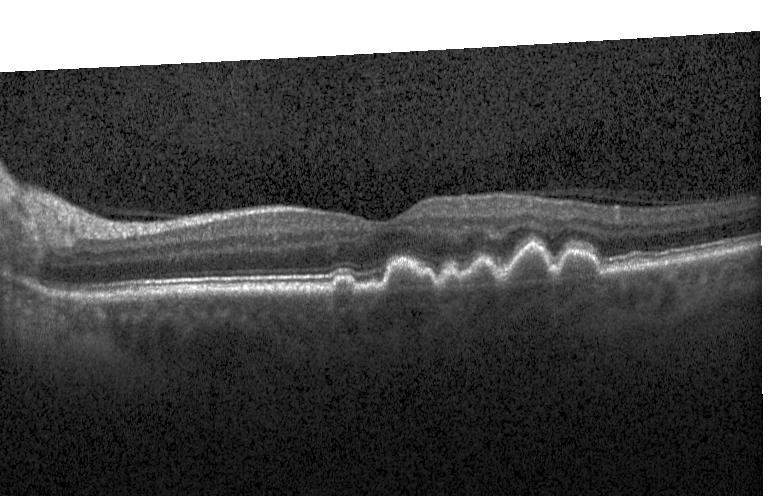 Finding: drusen.